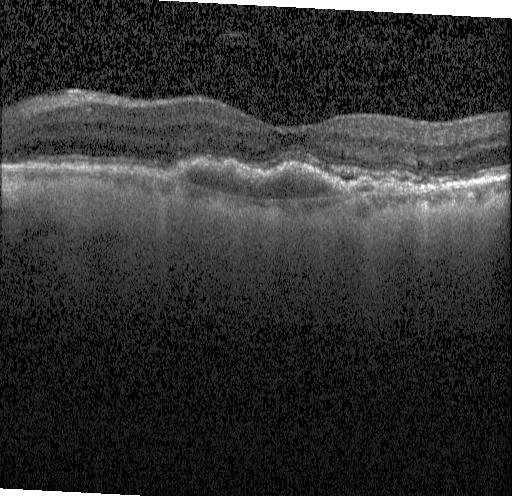

This B-scan demonstrates a choroidal neovascular membrane.